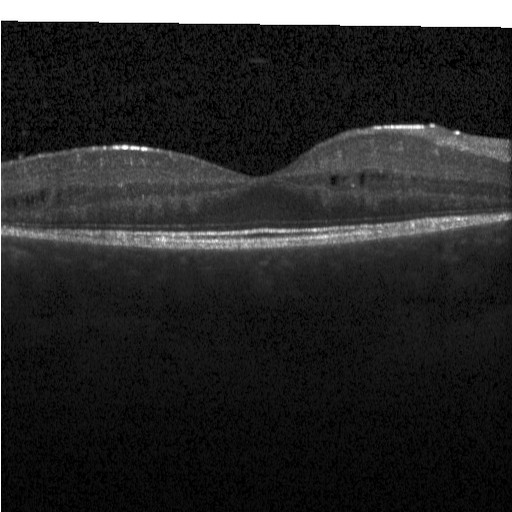

Retinal OCT cross-section.
Dx: diabetic macular edema.